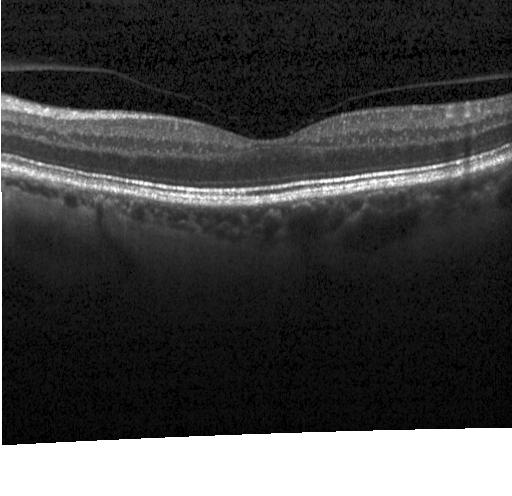
Impression: neither CNV, DME, nor drusen.